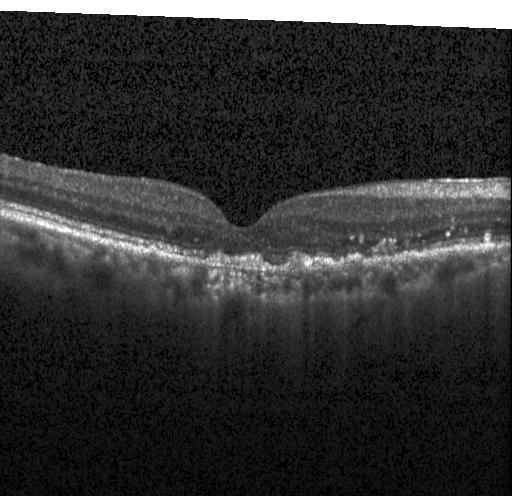

Spectral-domain optical coherence tomography; Heidelberg Spectralis OCT system; optical coherence tomography scan; horizontal scan through the fovea — Macular OCT: a choroidal neovascular membrane.